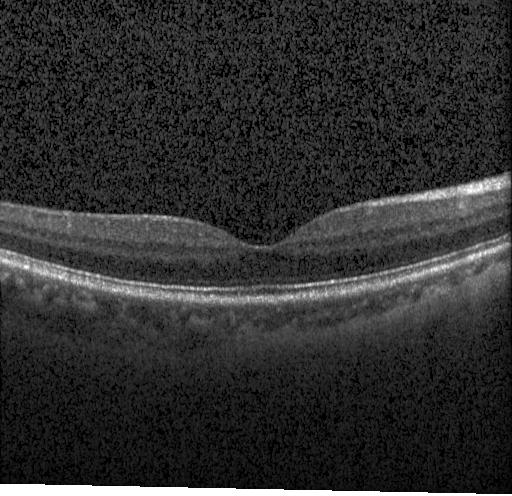
Heidelberg Spectralis, OCT B-scan, SD-OCT. Dx: no choroidal neovascularization, no diabetic macular edema, and no drusen.